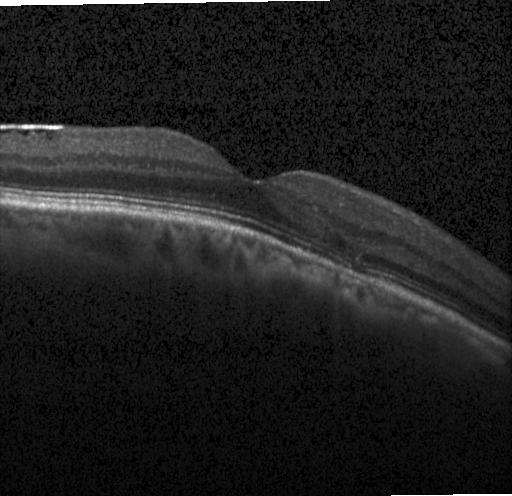

Macular OCT: no evidence of choroidal neovascularization, diabetic macular edema, or drusen.